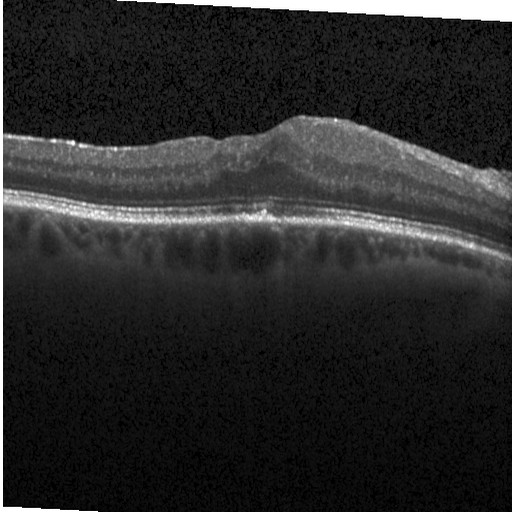

Instrument: Heidelberg Spectralis · SD-OCT · through the macula · OCT line scan. Dx: diabetic macular edema (DME).